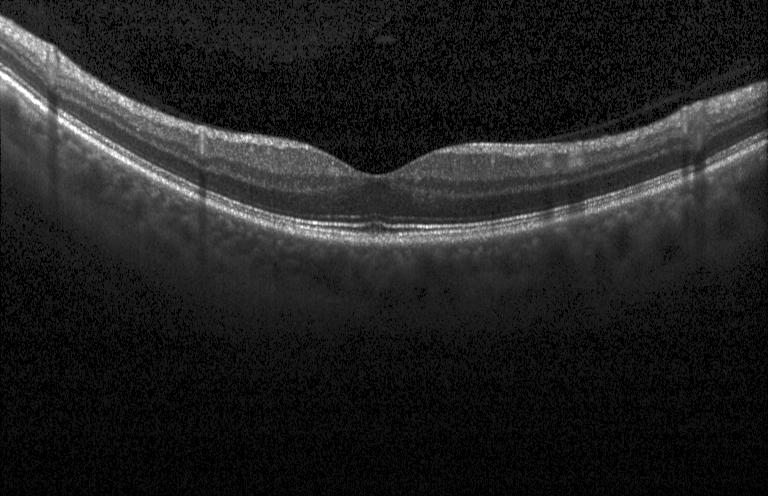

Assessment: no CNV, DME, or drusen.